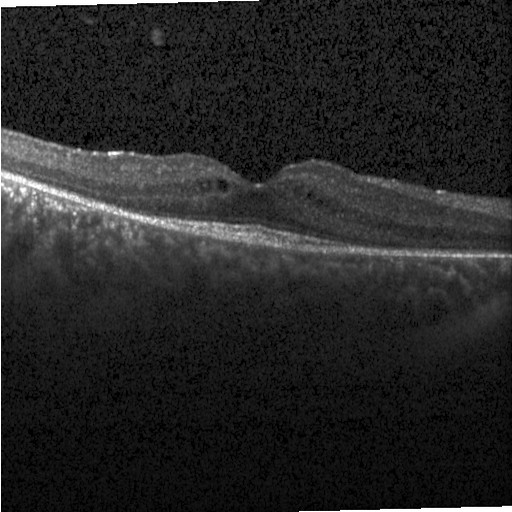
Spectral-domain optical coherence tomography. Retinal OCT cross-section — Assessment: diabetic macular edema.